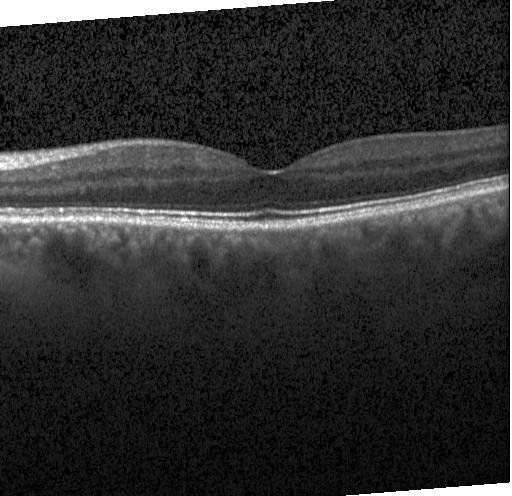 Dx: no evidence of choroidal neovascularization, diabetic macular edema, or drusen.